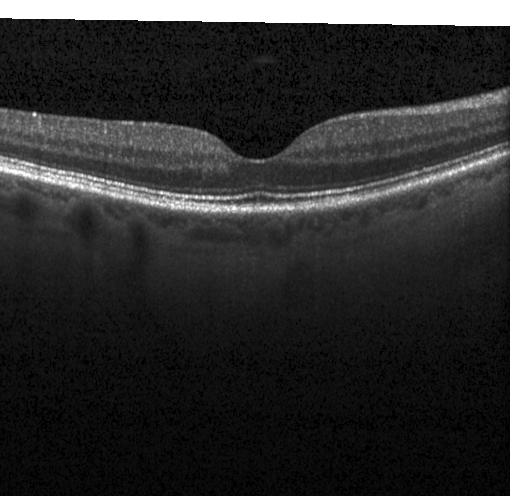 OCT finding: neither CNV, DME, nor drusen.